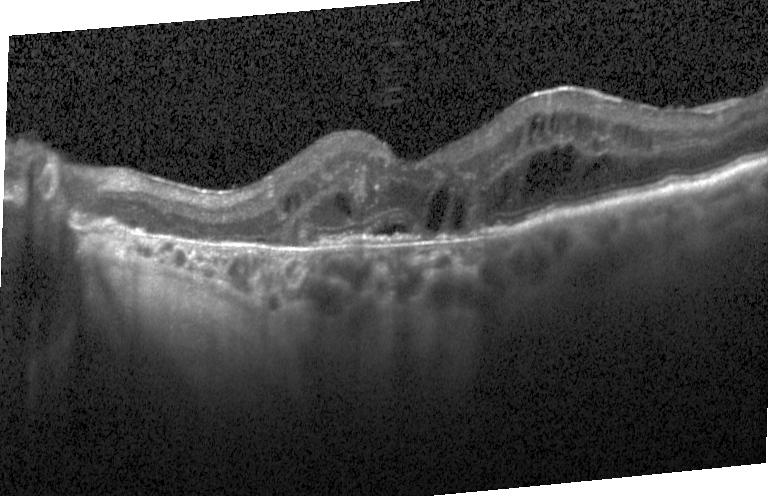
OCT finding: a choroidal neovascular membrane.